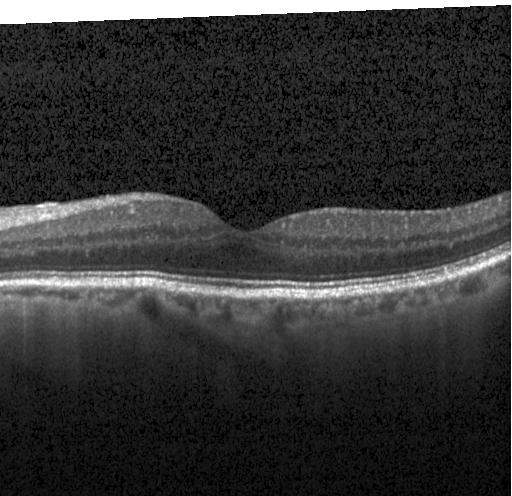
Heidelberg Spectralis OCT system · optical coherence tomography scan.
Diagnosis: no evidence of choroidal neovascularization, diabetic macular edema, or drusen.